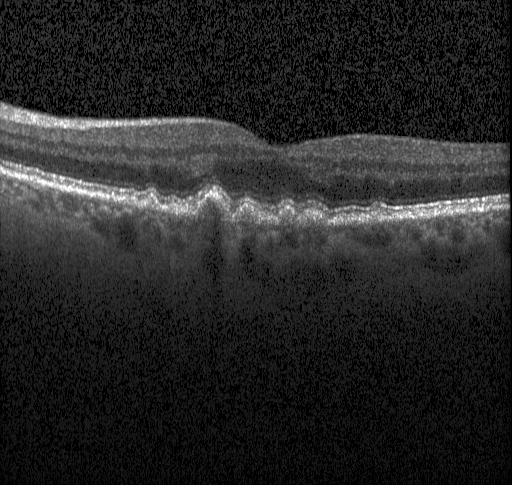
Retinal OCT cross-section showing sub-RPE drusenoid deposits.